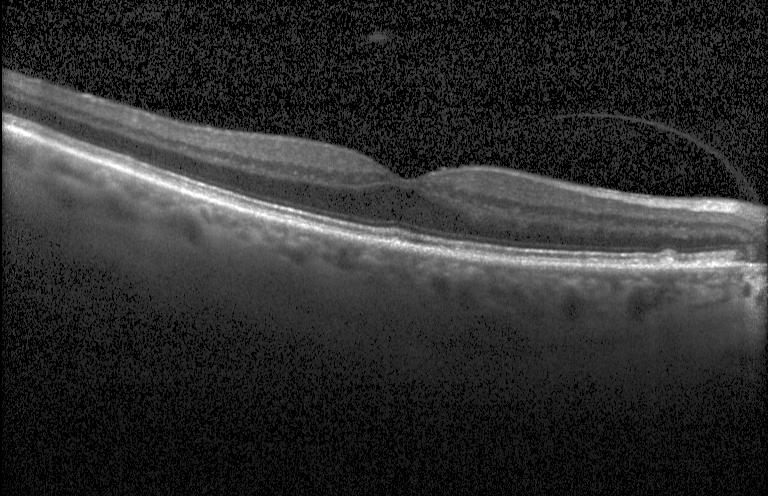
Finding: drusen.